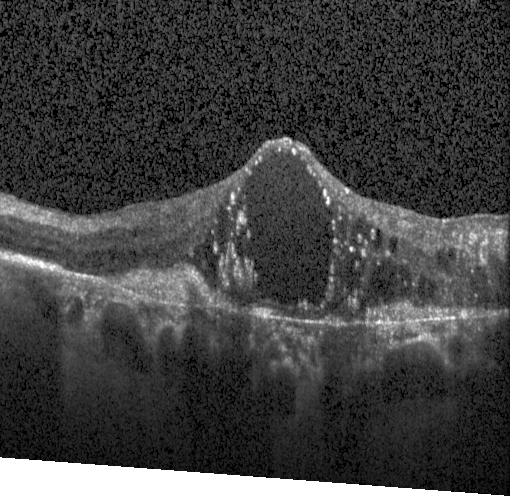
Finding: CNV.